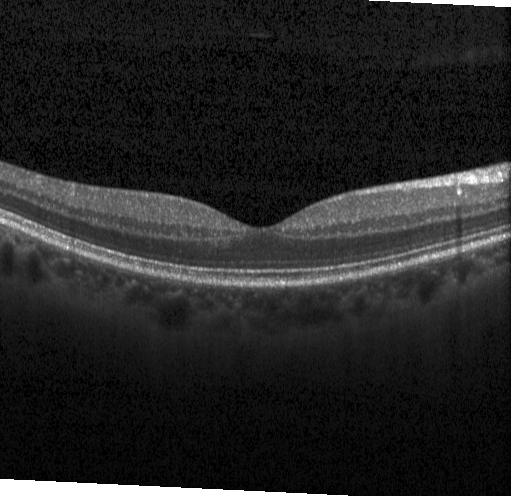
Optical coherence tomography scan · instrument: Heidelberg Spectralis. OCT finding: no choroidal neovascularization, no diabetic macular edema, and no drusen.